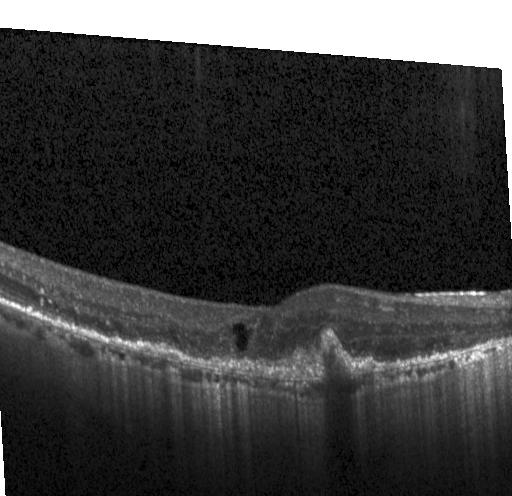

Retinal OCT cross-section. OCT finding: a choroidal neovascular membrane.